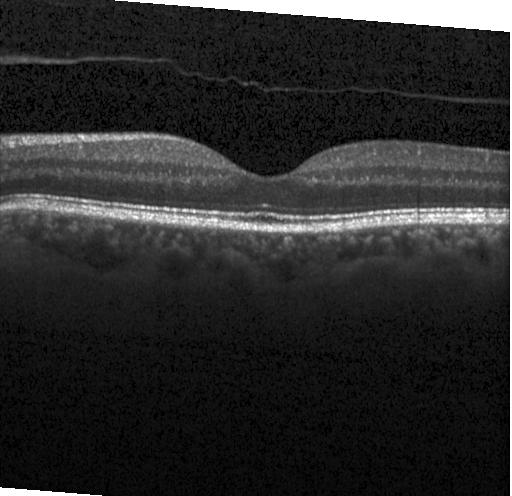
Optical coherence tomography B-scan.
Macular OCT: no choroidal neovascularization, diabetic macular edema, or drusen.